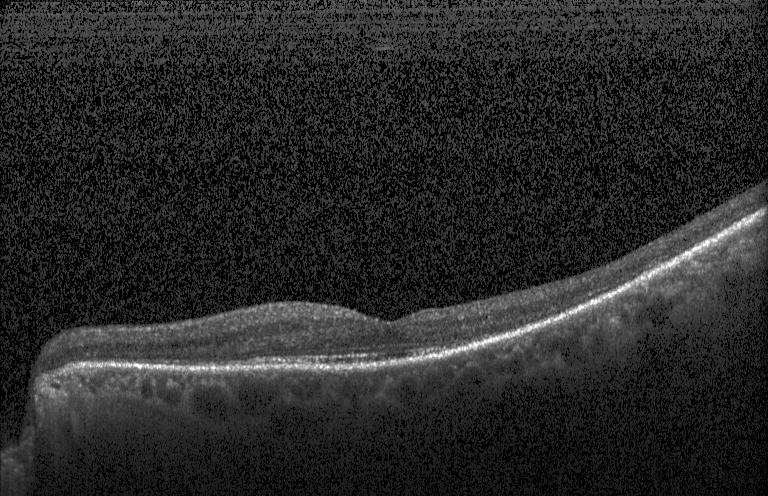

Dx: no choroidal neovascularization, diabetic macular edema, or drusen.